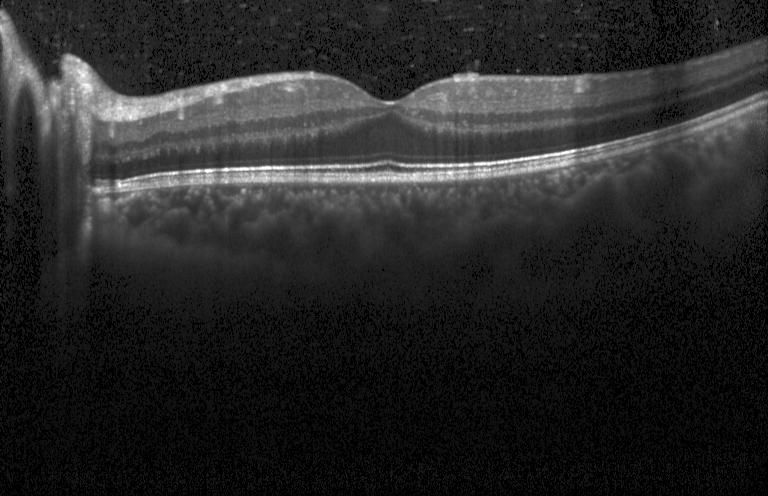

Spectral-domain OCT B-scan: no CNV, no DME, and no drusen.